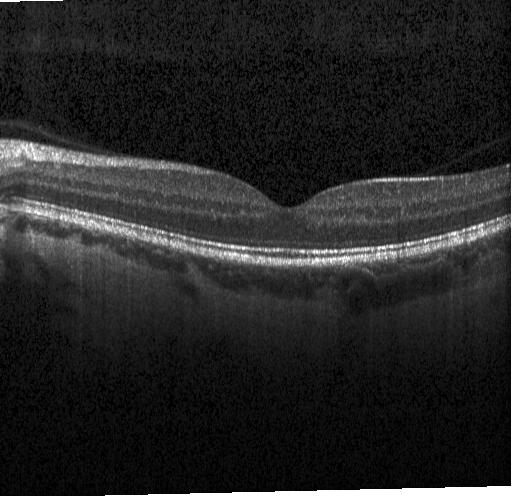

Diagnosis: no choroidal neovascularization, diabetic macular edema, or drusen.